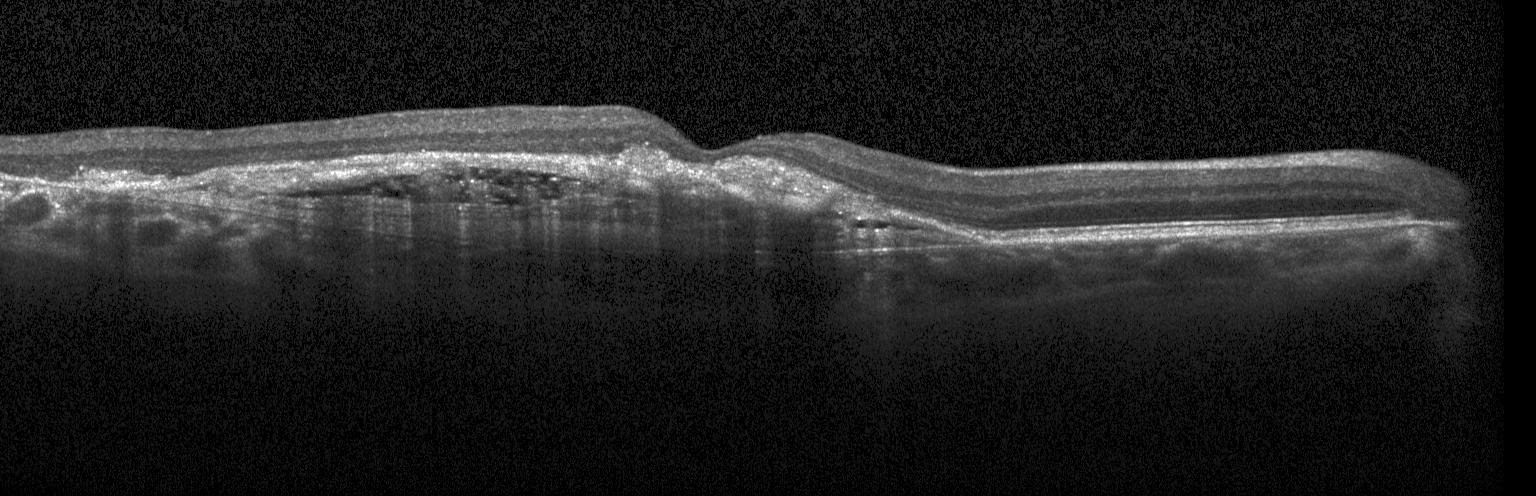
Retinal OCT cross-section.
Assessment: choroidal neovascularization.